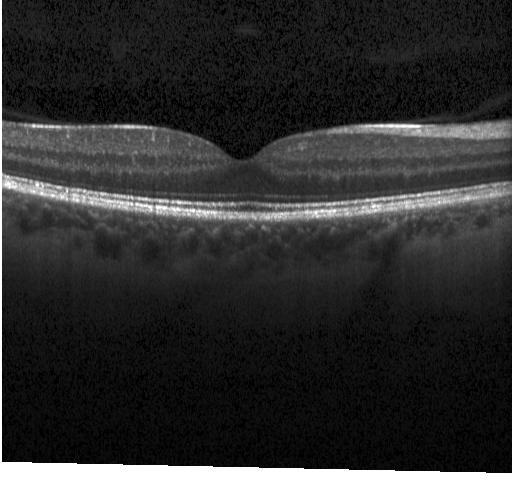 Impression: no CNV, DME, or drusen.